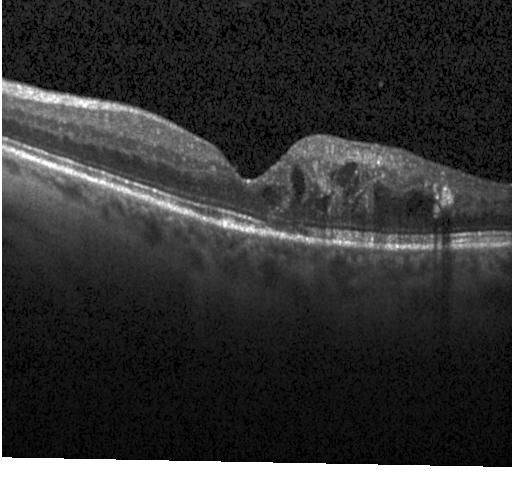

OCT line scan
Impression: diabetic macular edema.